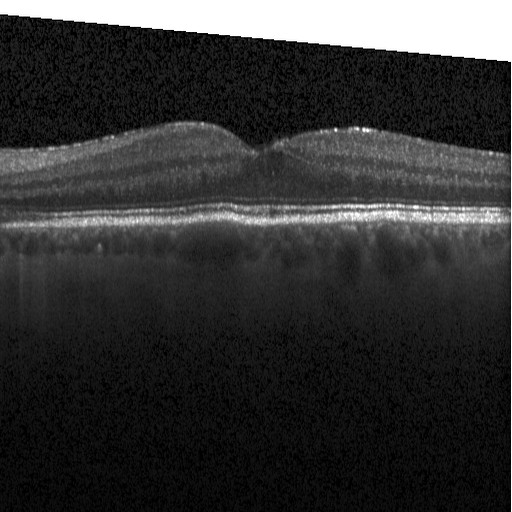

Spectral-domain OCT, optical coherence tomography B-scan, fovea-centered, Heidelberg Spectralis OCT system. OCT finding: DME.